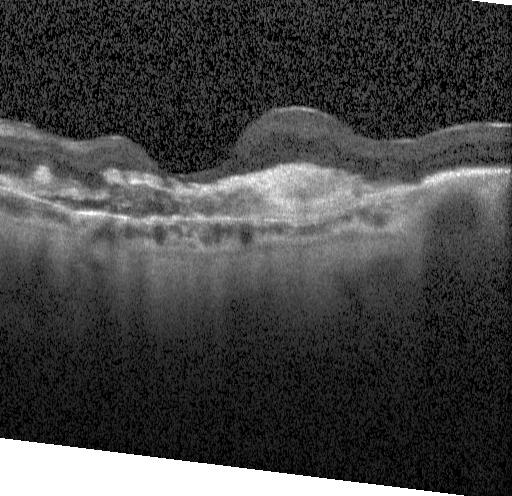 Spectral-domain OCT; OCT line scan. Choroidal neovascularization (CNV).